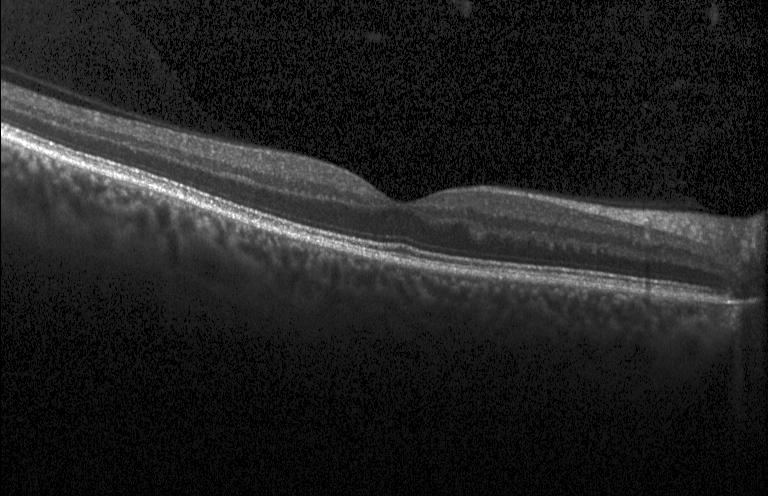
Centered on the fovea · SD-OCT · acquired on a Heidelberg Spectralis · retinal OCT B-scan — Assessment: neither CNV, DME, nor drusen.